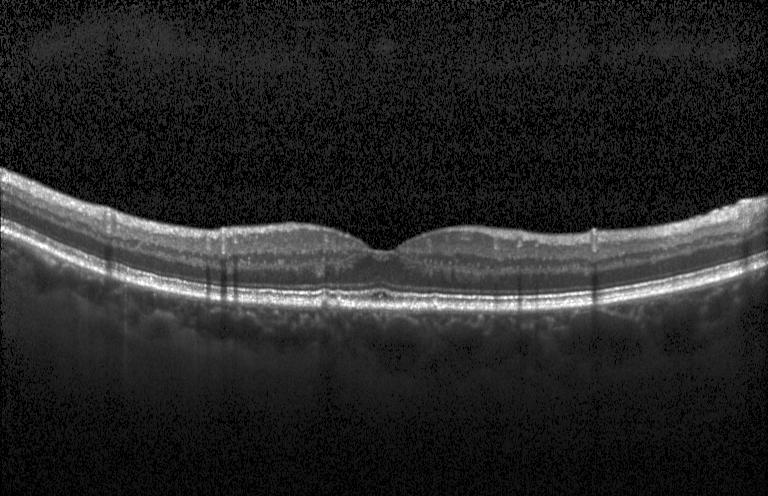 Diagnosis: drusen.